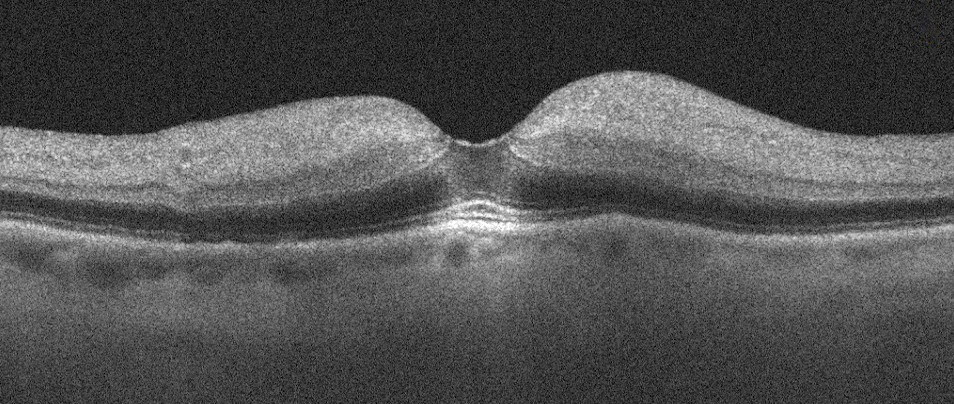
Retinal OCT cross-section showing RAO.